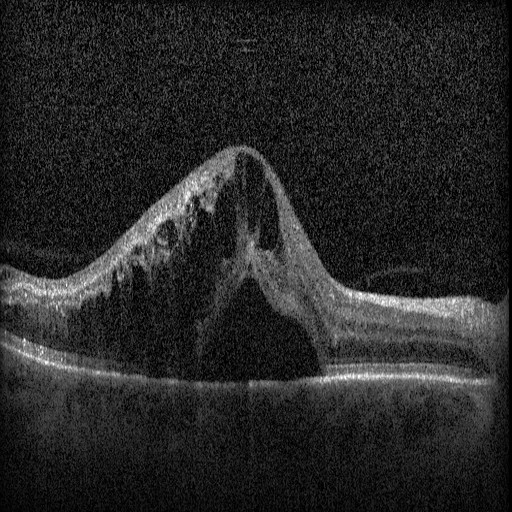 Retinal OCT cross-section showing DME.